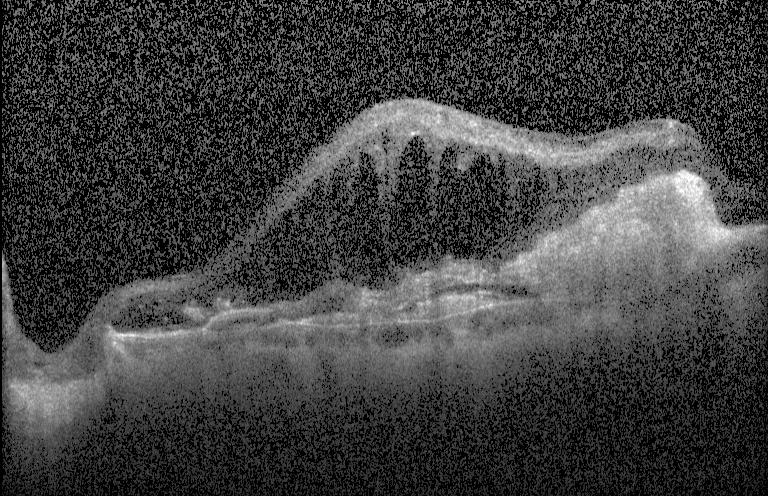

Heidelberg Spectralis OCT system, fovea-centered, optical coherence tomography B-scan.
Finding: a choroidal neovascular membrane.